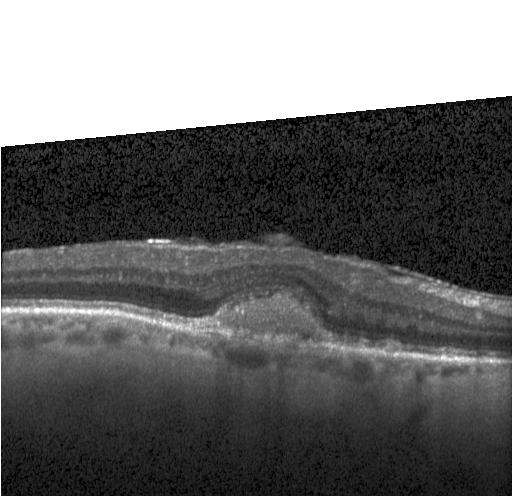
Impression: choroidal neovascularization.